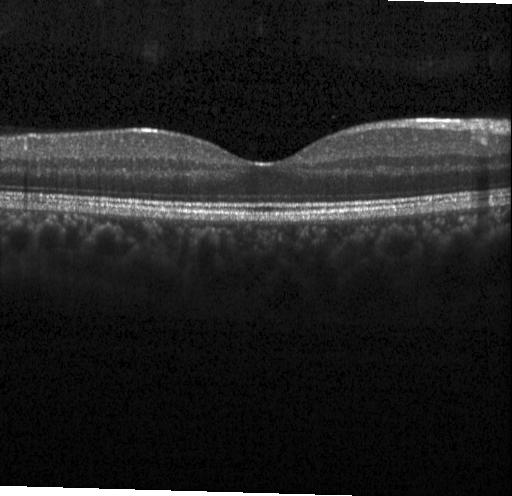 Acquired on a Heidelberg Spectralis; SD-OCT; centered on the fovea; retinal OCT cross-section — Impression: no evidence of CNV, DME, or drusen.